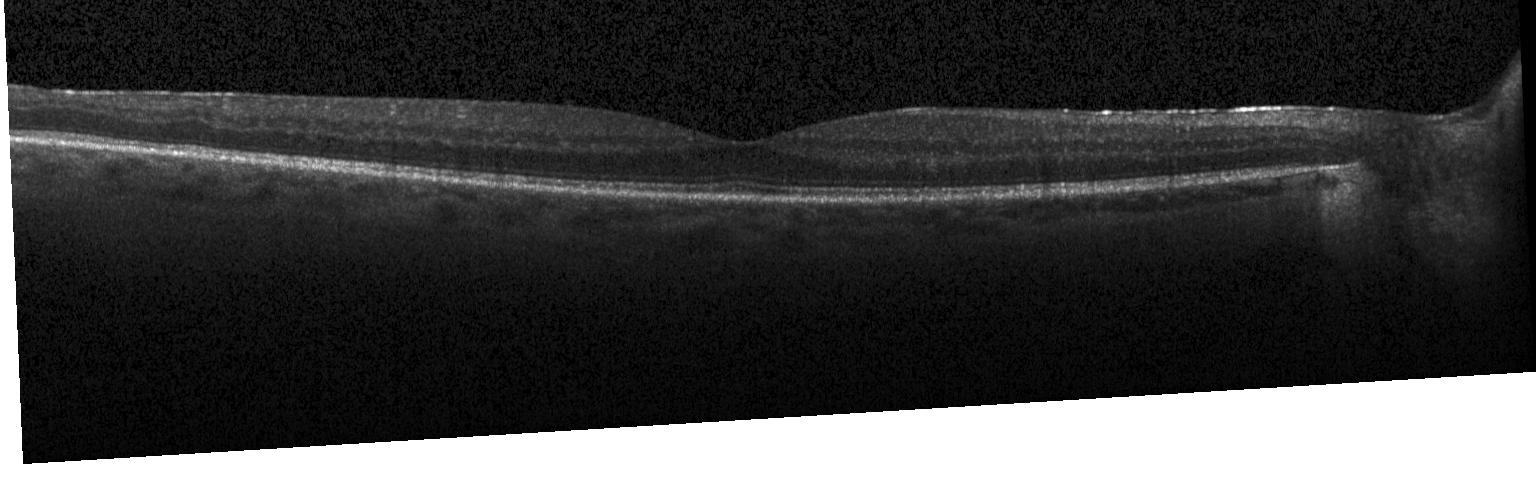
Spectral-domain optical coherence tomography. Retinal OCT B-scan.
Neither choroidal neovascularization, diabetic macular edema, nor drusen.